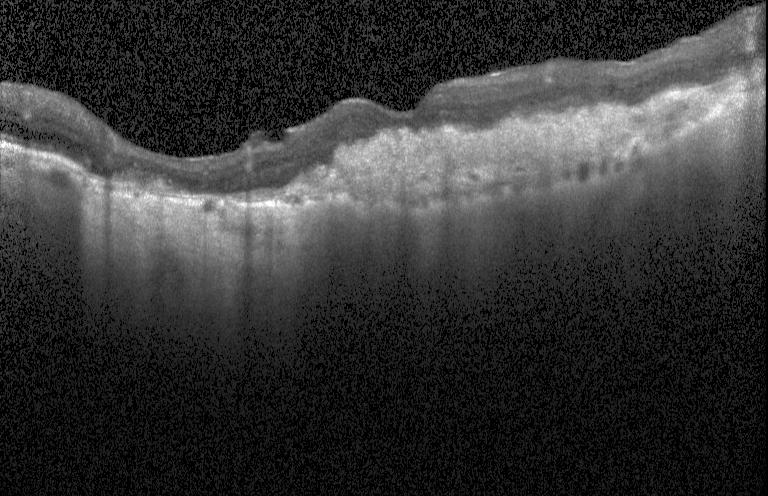

Finding: a choroidal neovascular membrane.